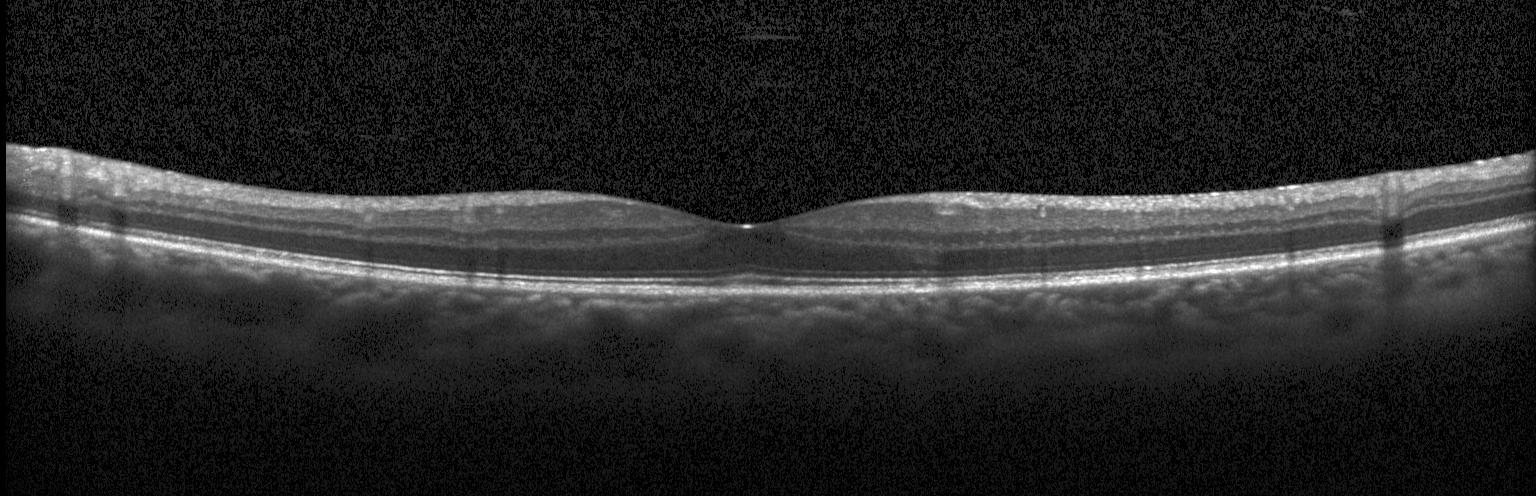

OCT finding: no evidence of CNV, DME, or drusen.